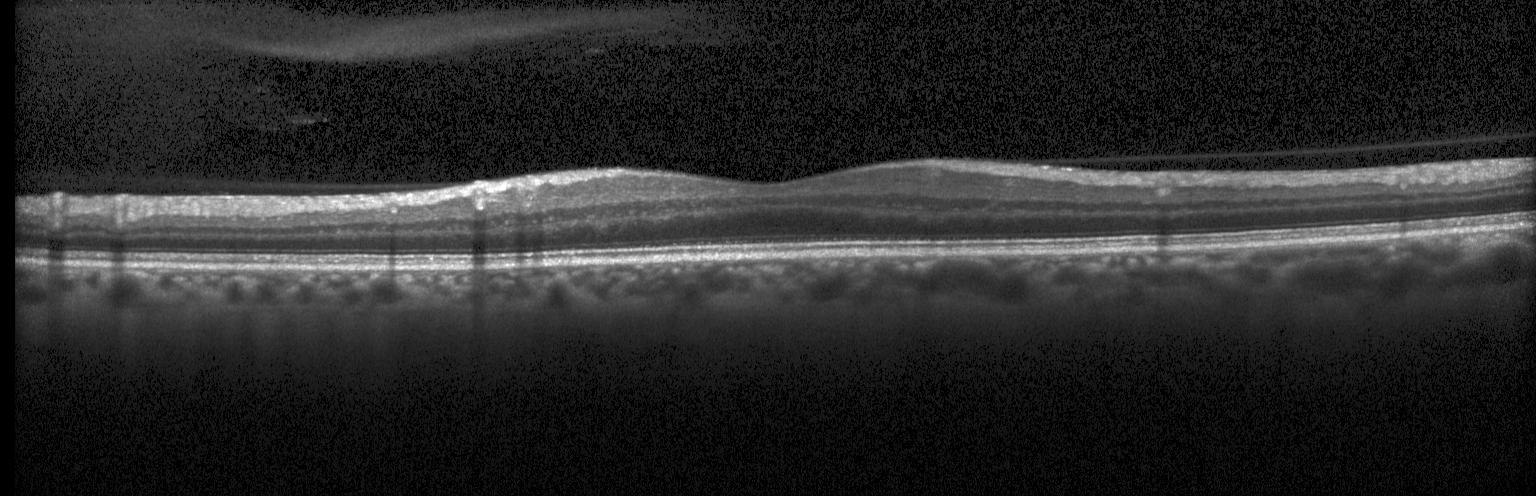
Acquired on a Heidelberg Spectralis · OCT line scan · horizontal scan through the fovea. Macular OCT: neither choroidal neovascularization, diabetic macular edema, nor drusen.